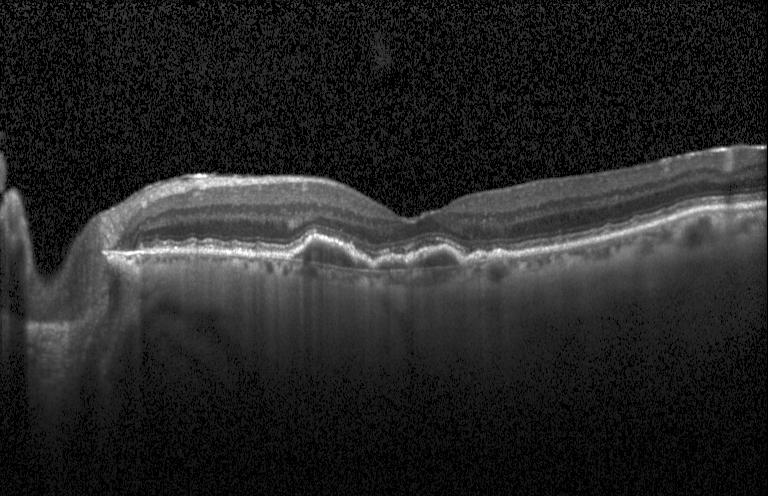
OCT B-scan showing a choroidal neovascular membrane.